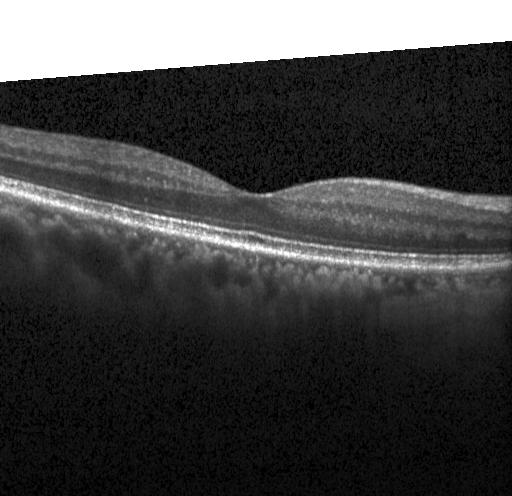
Finding: no choroidal neovascularization, no diabetic macular edema, and no drusen.